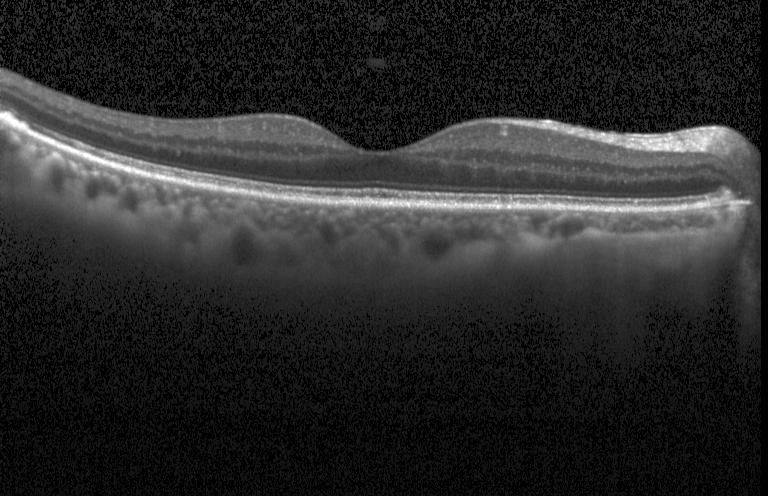 Assessment: no choroidal neovascularization, no diabetic macular edema, and no drusen.